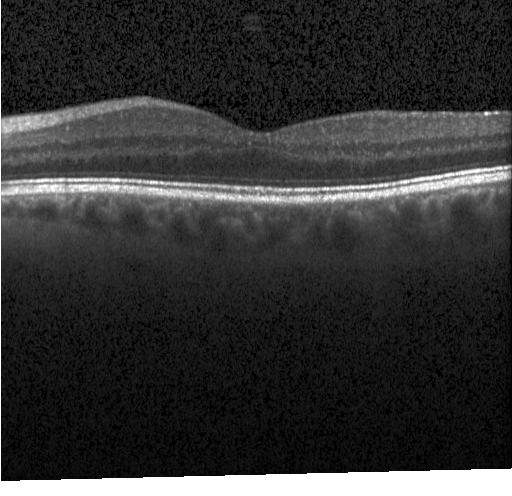

Impression: no evidence of CNV, DME, or drusen.